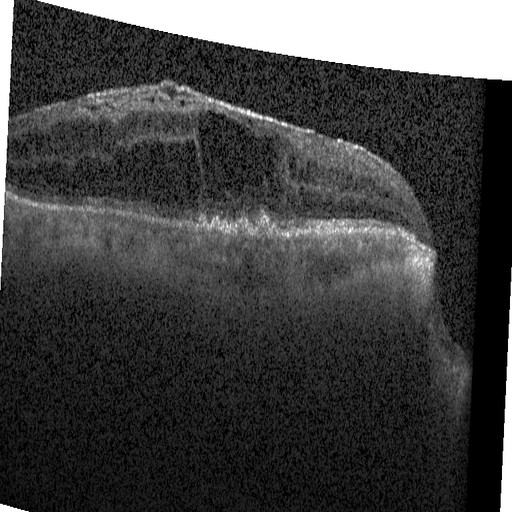

Retinal OCT cross-section — Impression: diabetic macular edema (DME).